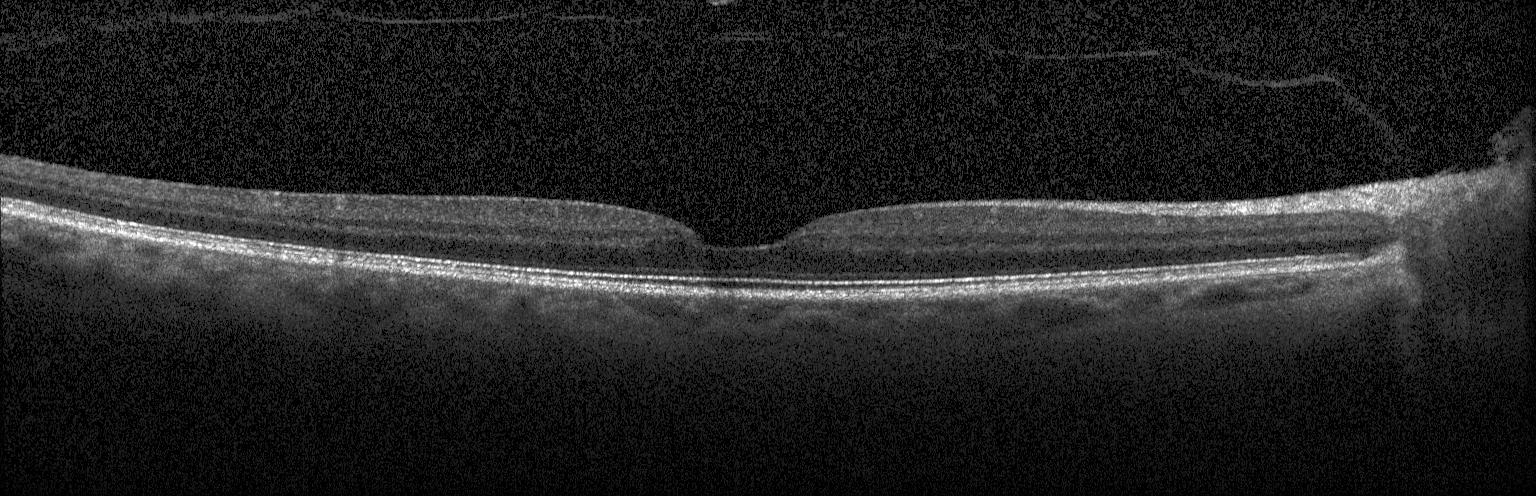
OCT scan showing neither choroidal neovascularization, diabetic macular edema, nor drusen.